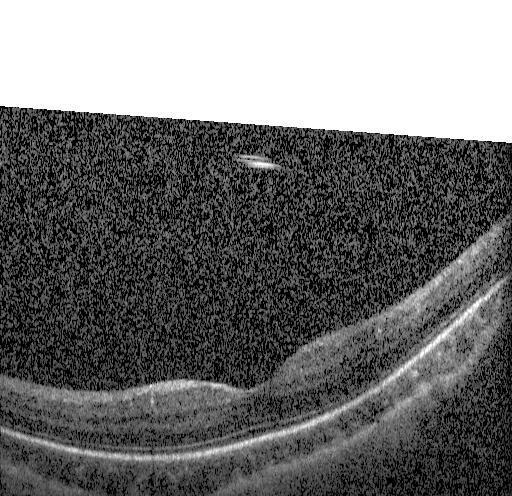 This B-scan demonstrates neither choroidal neovascularization, diabetic macular edema, nor drusen.